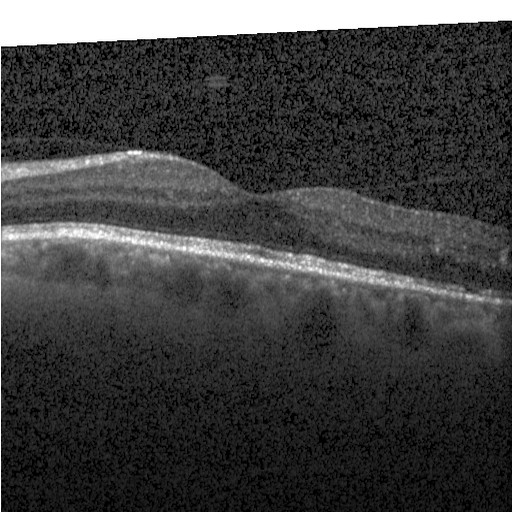
OCT B-scan. Heidelberg Spectralis. Spectral-domain OCT. Through the macula. Diagnosis: DME.